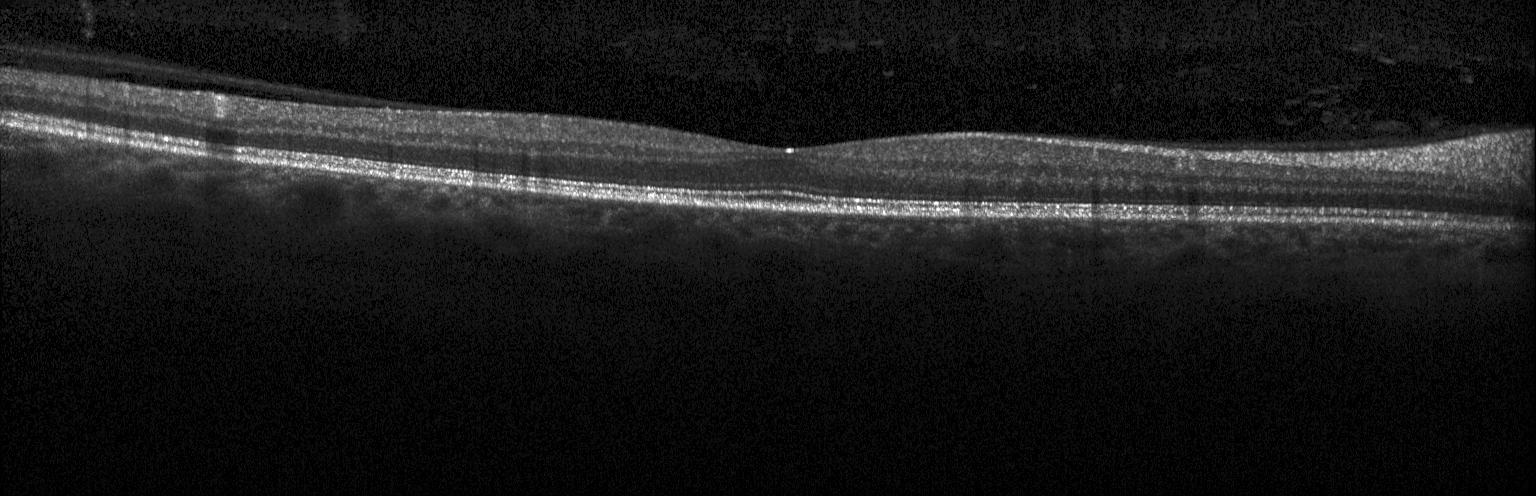
OCT B-scan showing no CNV, no DME, and no drusen.